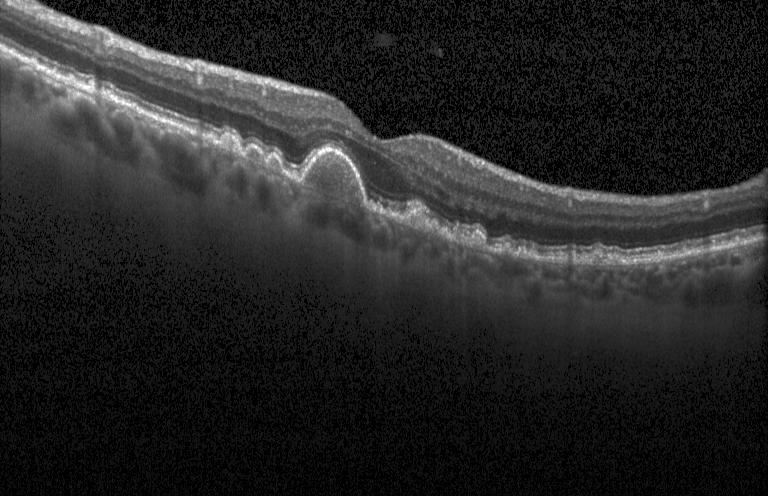
Instrument: Heidelberg Spectralis; retinal OCT cross-section; spectral-domain optical coherence tomography; horizontal scan through the fovea — Finding: drusen.